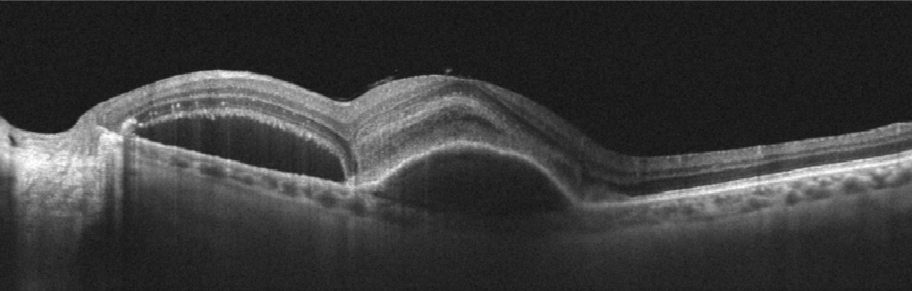

Optical coherence tomography B-scan · fovea-centered · acquired on an Optovue Avanti RTVue XR — Age-related macular degeneration.